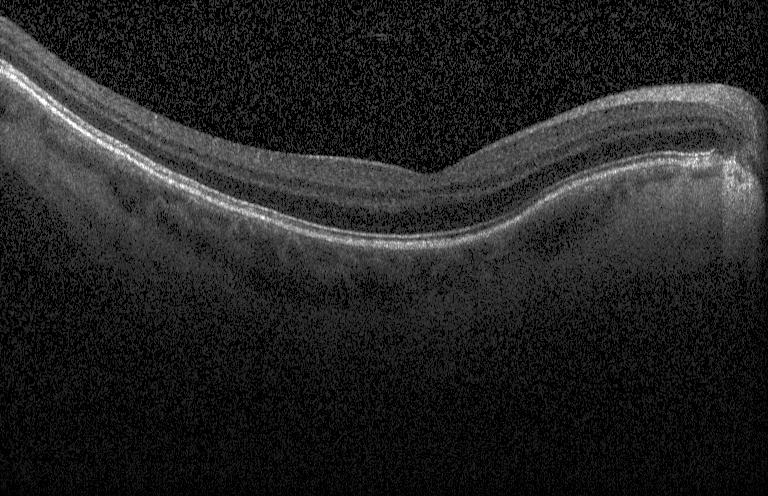 Dx: no choroidal neovascularization, no diabetic macular edema, and no drusen.